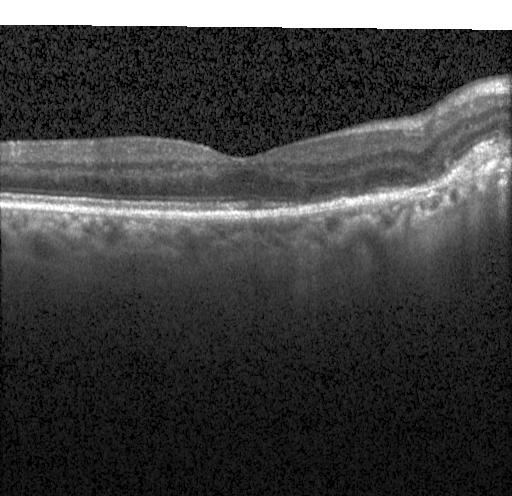
OCT line scan. Dx: choroidal neovascularization (CNV).